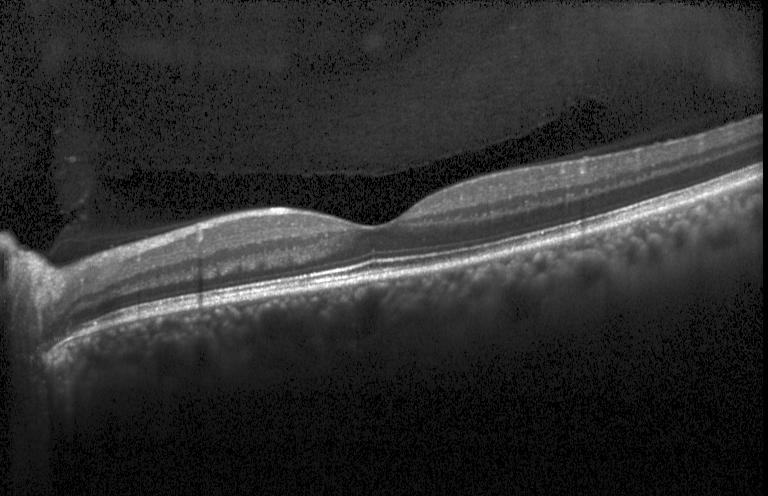 OCT line scan. Diagnosis: no choroidal neovascularization, no diabetic macular edema, and no drusen.